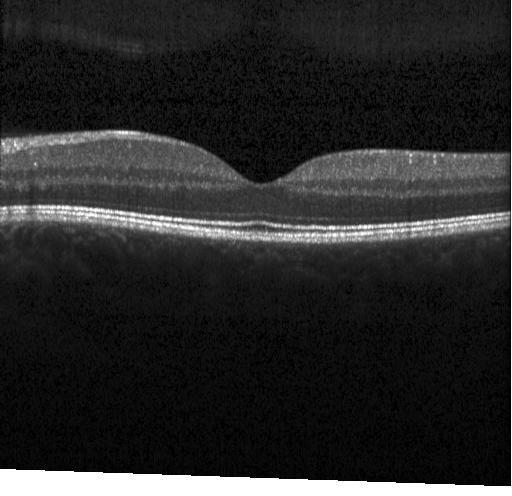

Heidelberg Spectralis OCT system, OCT B-scan
Dx: no CNV, DME, or drusen.